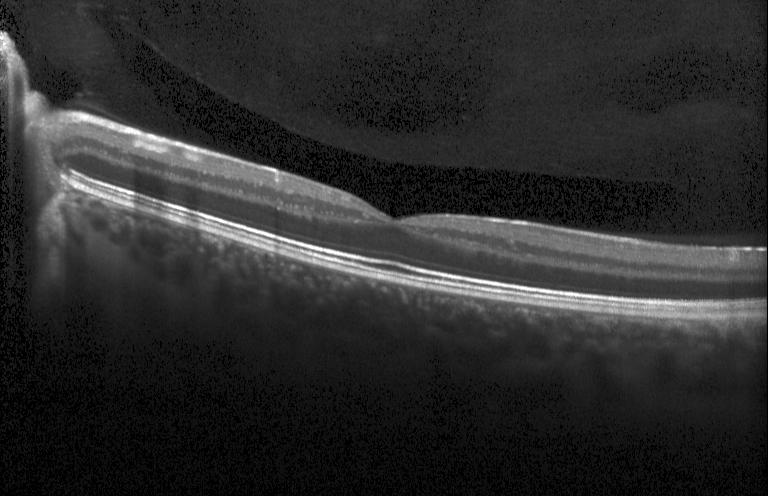 Optical coherence tomography scan. Diagnosis: no evidence of CNV, DME, or drusen.